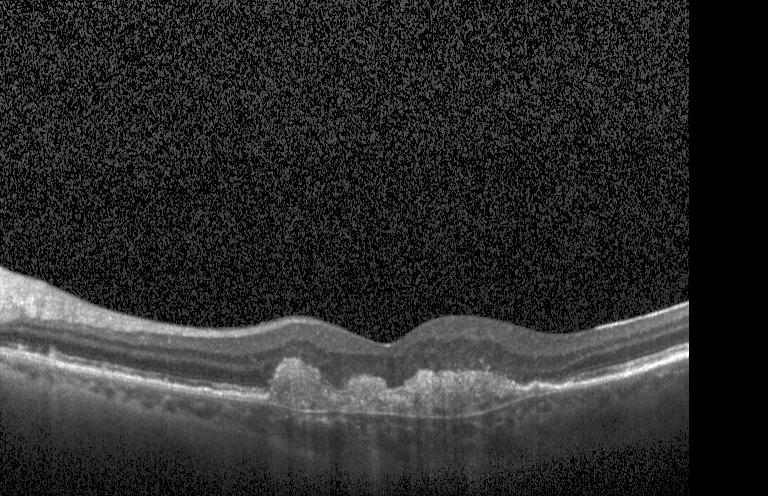
Finding: choroidal neovascularization.